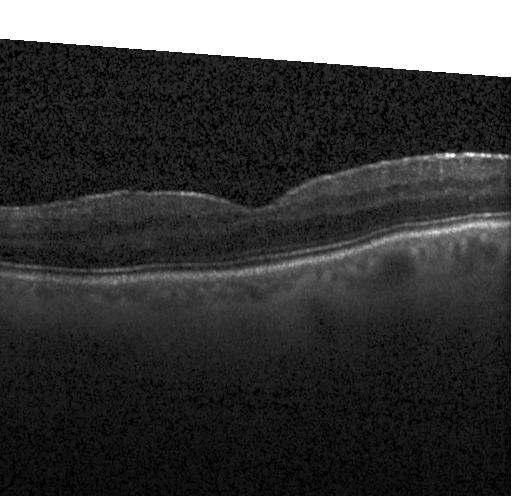

Through the macula, Heidelberg Spectralis OCT system, SD-OCT, OCT line scan — Macular OCT: no evidence of choroidal neovascularization, diabetic macular edema, or drusen.